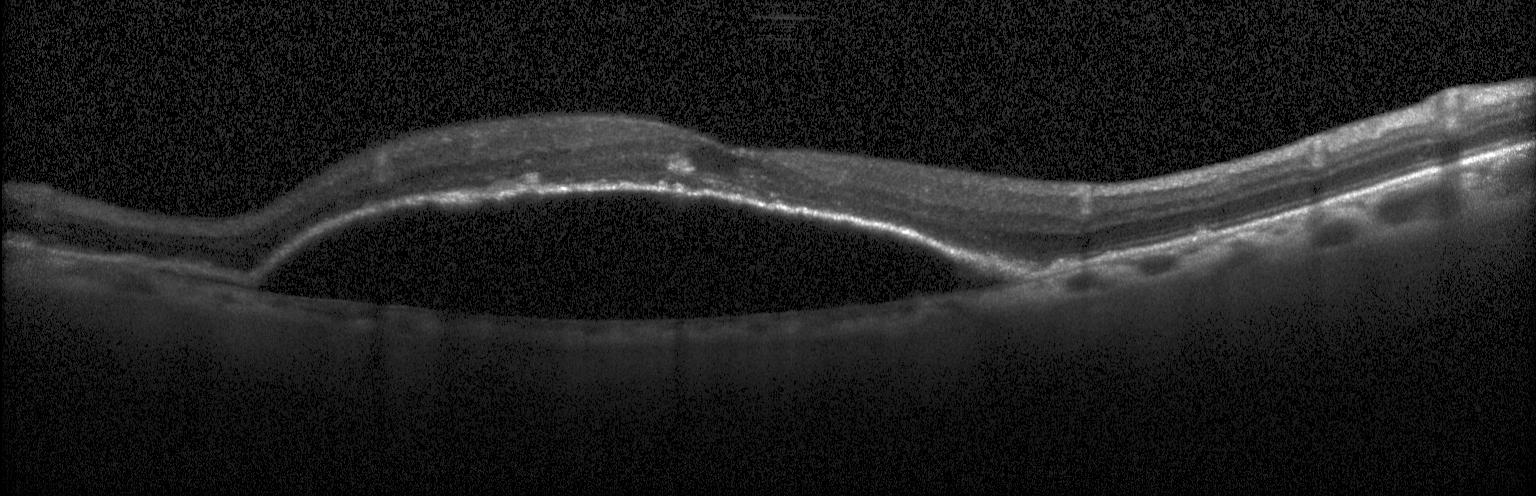
Macular OCT: a choroidal neovascular membrane.